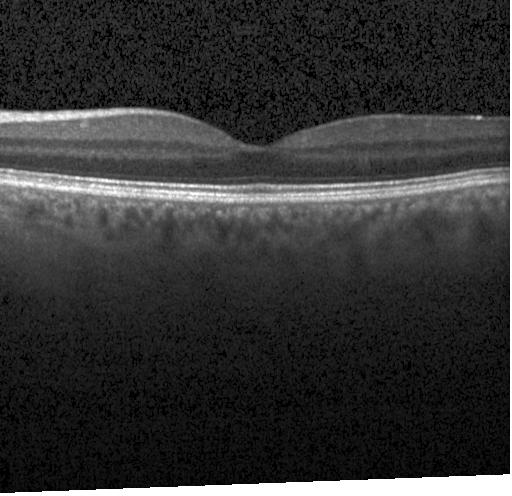

Spectral-domain OCT B-scan: no choroidal neovascularization, diabetic macular edema, or drusen.